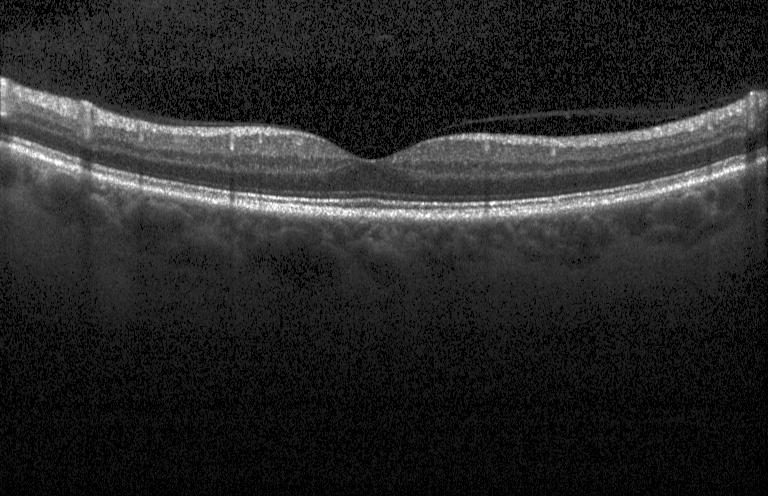 Dx: neither choroidal neovascularization, diabetic macular edema, nor drusen.